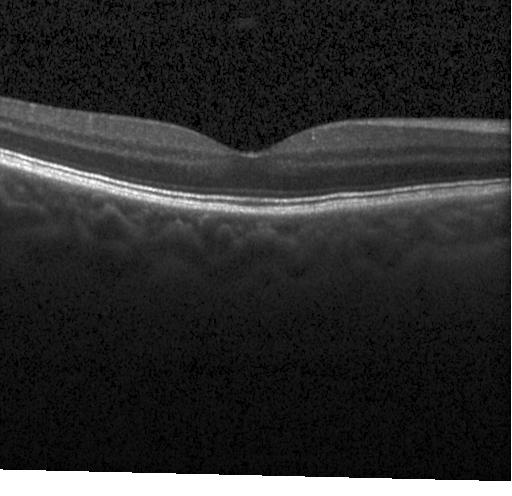

Retinal OCT cross-section — Finding: no CNV, no DME, and no drusen.